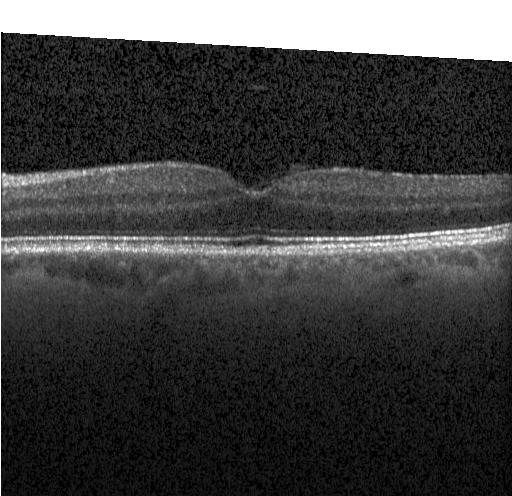

Instrument: Heidelberg Spectralis; retinal OCT cross-section; centered on the fovea. This B-scan demonstrates neither choroidal neovascularization, diabetic macular edema, nor drusen.